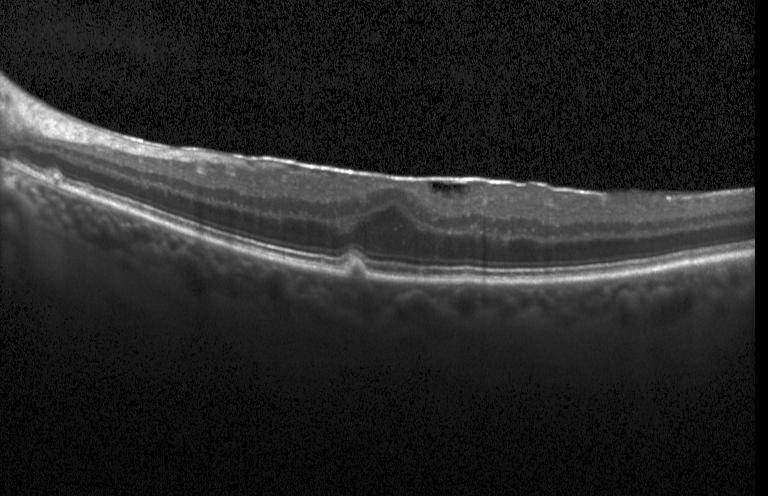
Dx: drusen.